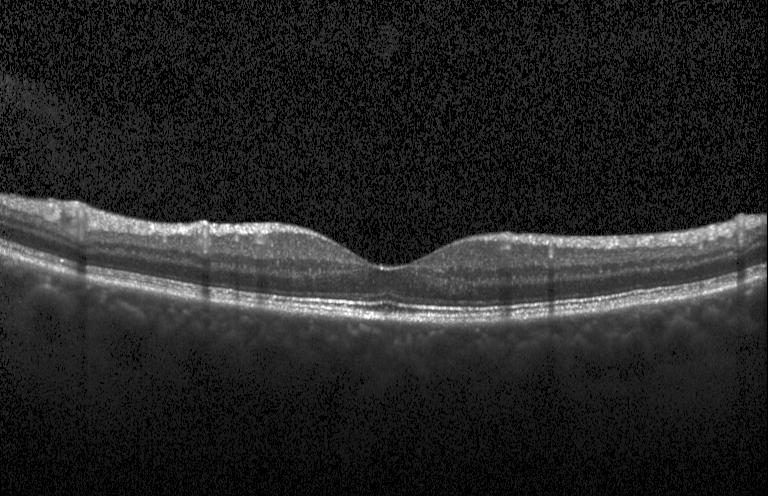
Macular OCT: neither CNV, DME, nor drusen.